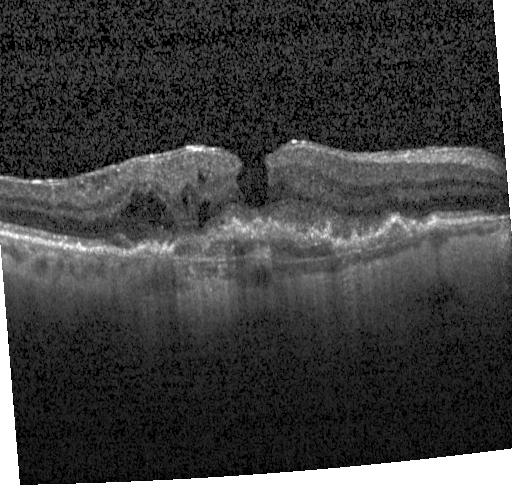 Macular OCT: a choroidal neovascular membrane.